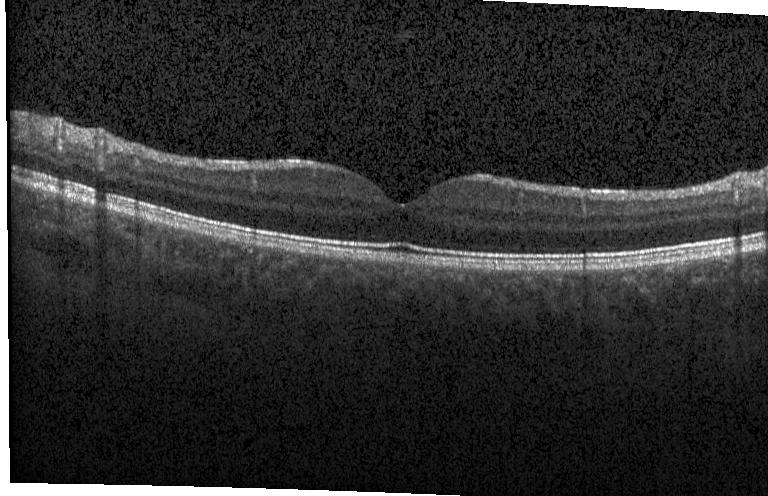 Dx: no CNV, DME, or drusen.